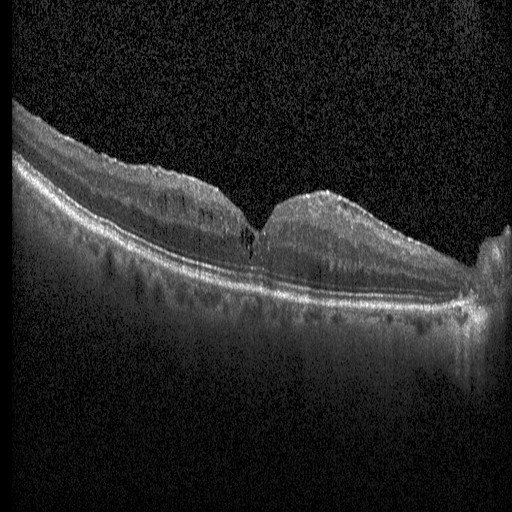

Diagnosis: diabetic macular edema.